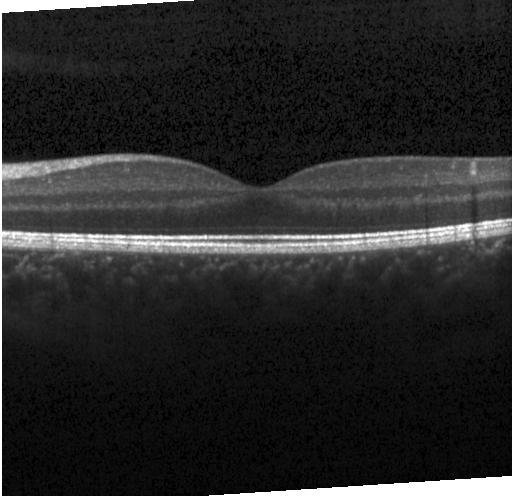

Finding: no CNV, no DME, and no drusen.